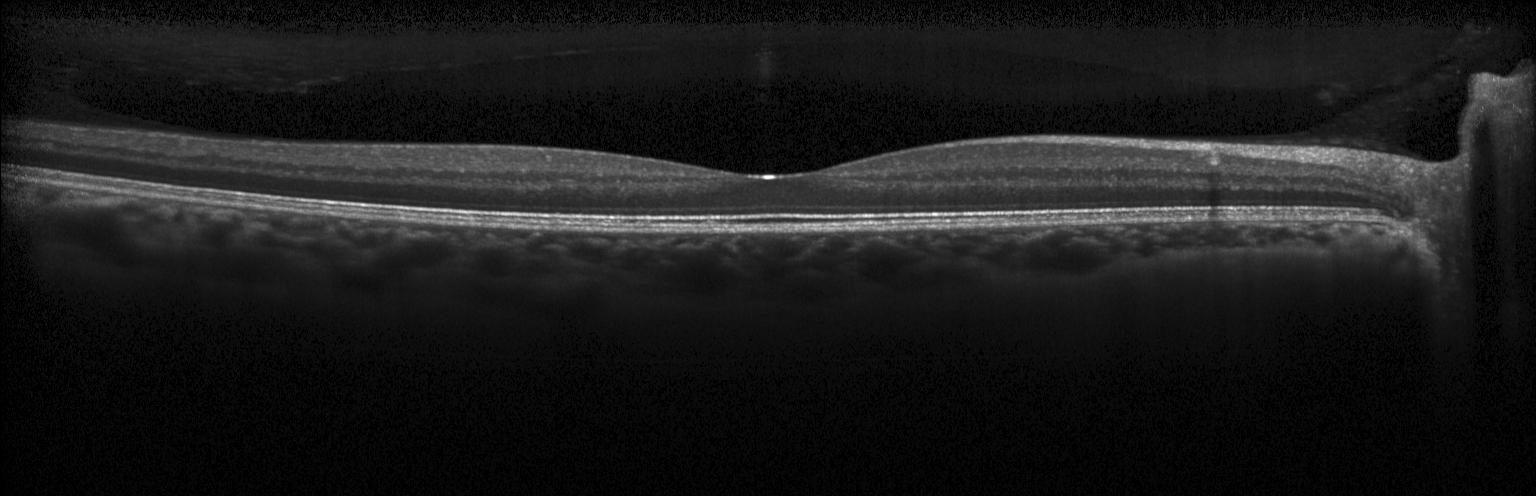
The scan shows no choroidal neovascularization, no diabetic macular edema, and no drusen.